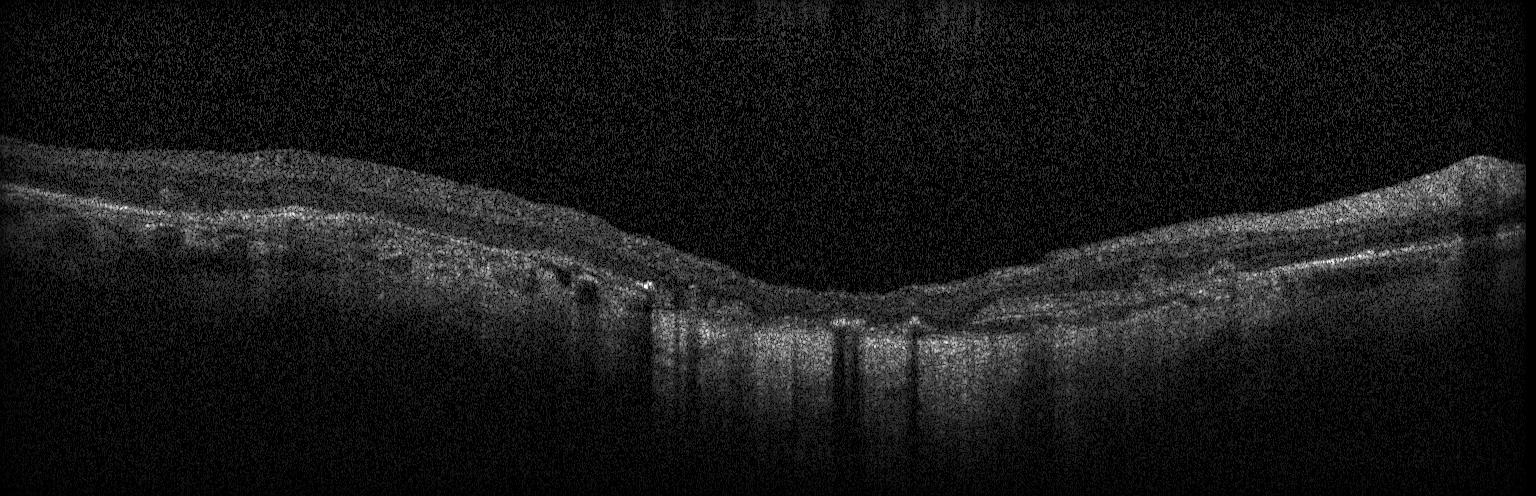

Optical coherence tomography scan · acquired on a Heidelberg Spectralis · horizontal scan through the fovea · spectral-domain OCT.
Finding: a choroidal neovascular membrane.